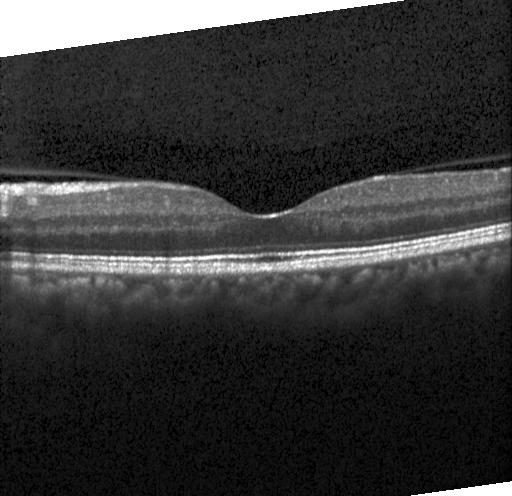
Heidelberg Spectralis OCT system; OCT B-scan; SD-OCT — Impression: neither choroidal neovascularization, diabetic macular edema, nor drusen.